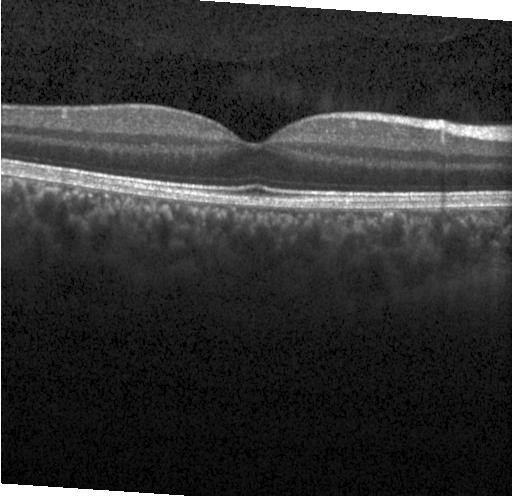
Retinal OCT cross-section — Dx: no choroidal neovascularization, diabetic macular edema, or drusen.